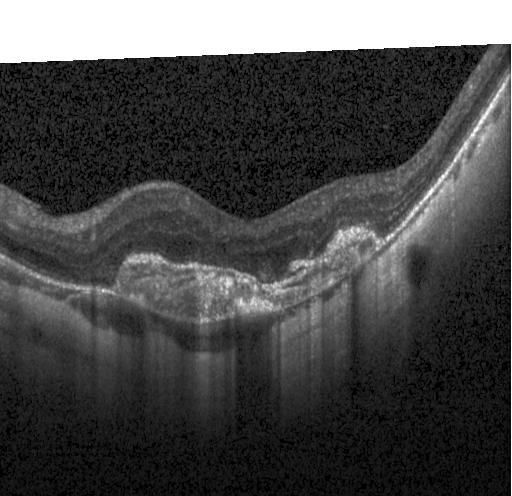

Heidelberg Spectralis · OCT line scan · spectral-domain OCT
OCT finding: a choroidal neovascular membrane.